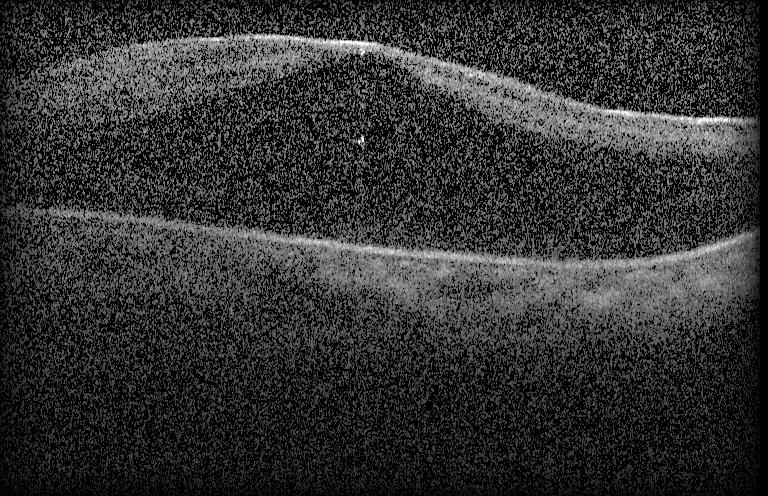
Impression: diabetic macular edema.